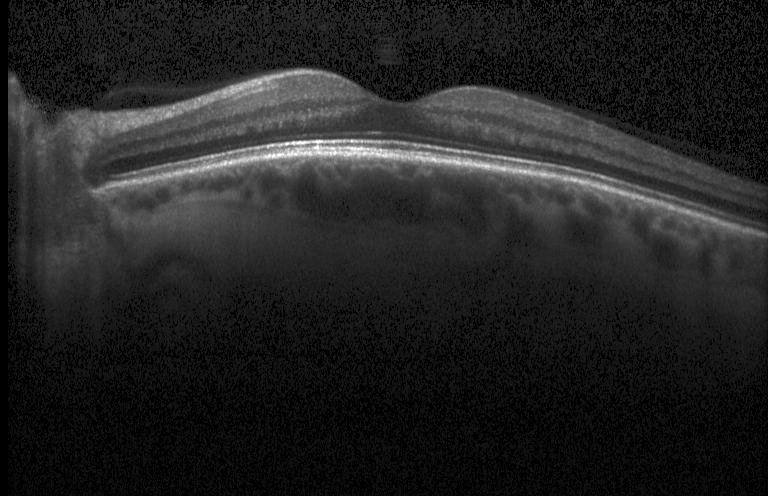 SD-OCT · OCT B-scan.
Macular OCT: no evidence of choroidal neovascularization, diabetic macular edema, or drusen.